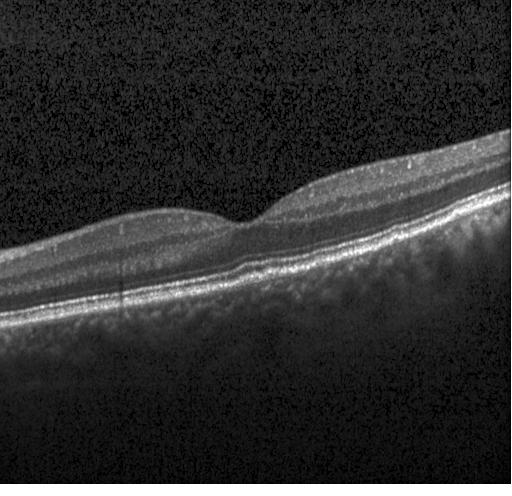
OCT finding: sub-RPE drusenoid deposits.